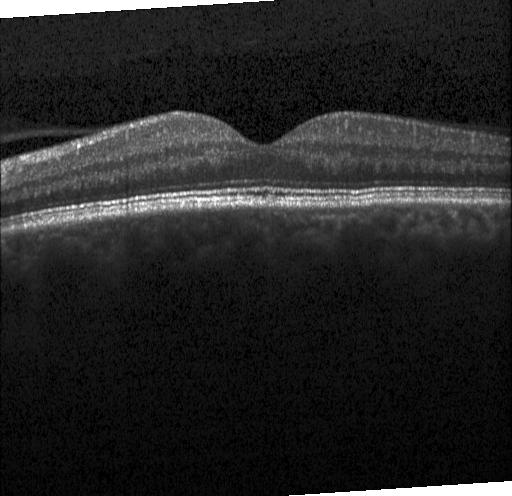

Impression: neither choroidal neovascularization, diabetic macular edema, nor drusen.